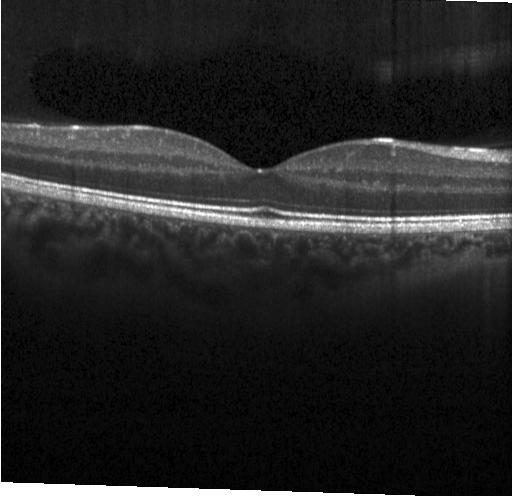

Heidelberg Spectralis; optical coherence tomography scan.
OCT finding: no evidence of CNV, DME, or drusen.